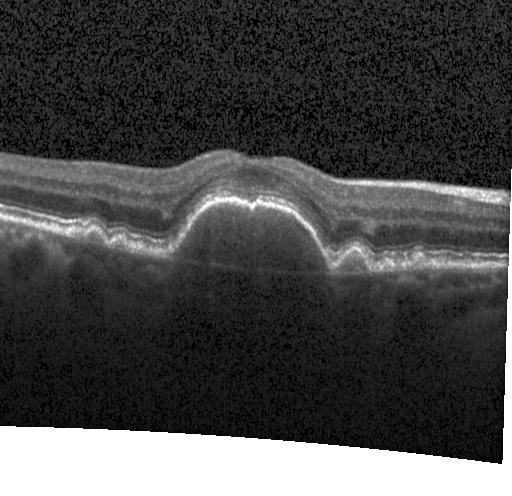 Acquired on a Heidelberg Spectralis · SD-OCT · OCT line scan · macular scan.
Macular OCT: choroidal neovascularization (CNV).